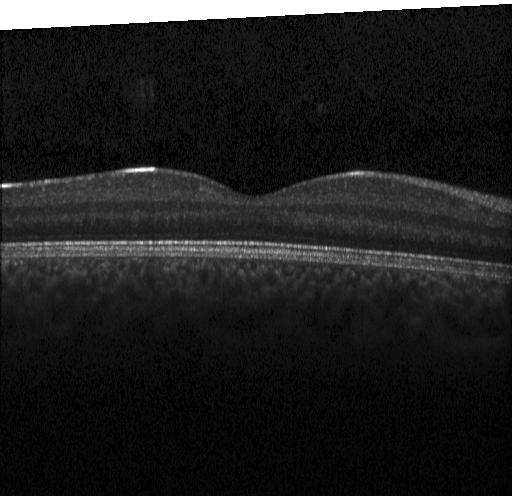 OCT finding: no evidence of choroidal neovascularization, diabetic macular edema, or drusen.